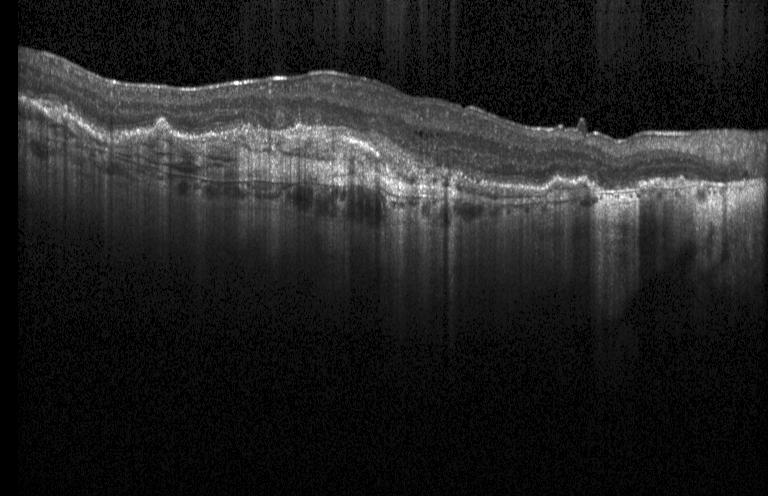

Diagnosis: a choroidal neovascular membrane.